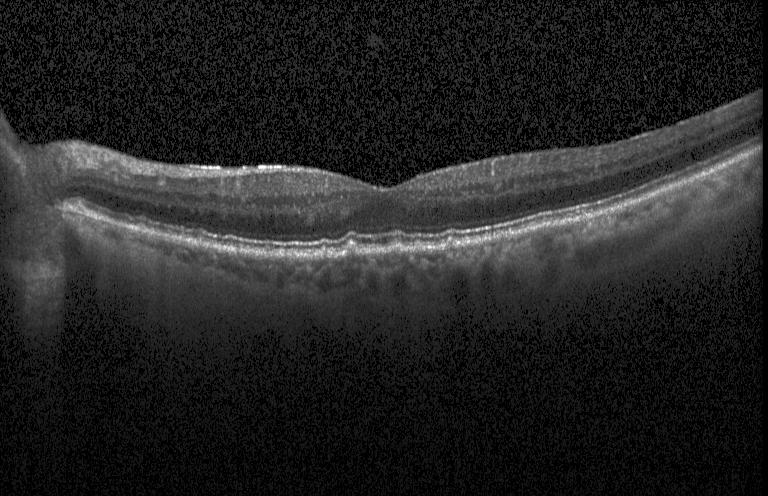

Through the macula. Heidelberg Spectralis. Spectral-domain optical coherence tomography. Optical coherence tomography scan
The scan shows drusen.